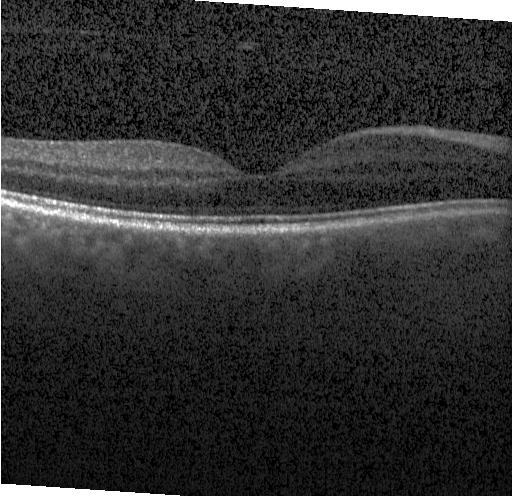
Finding: no choroidal neovascularization, diabetic macular edema, or drusen.